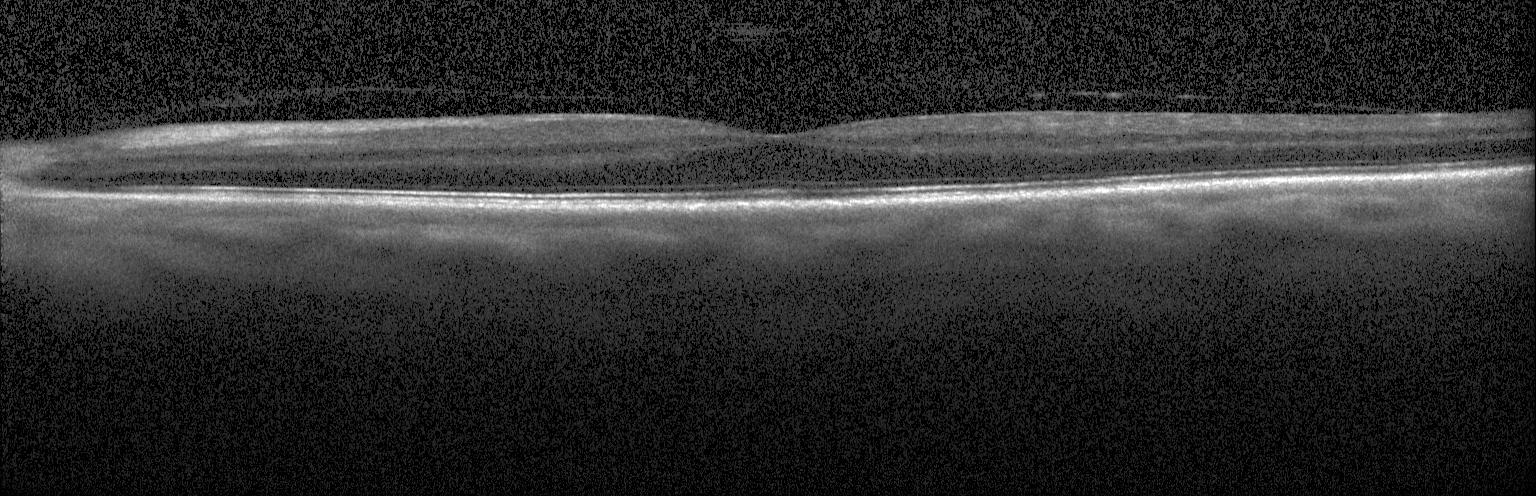 Optical coherence tomography B-scan · fovea-centered · spectral-domain OCT · Heidelberg Spectralis OCT system
Neither choroidal neovascularization, diabetic macular edema, nor drusen.